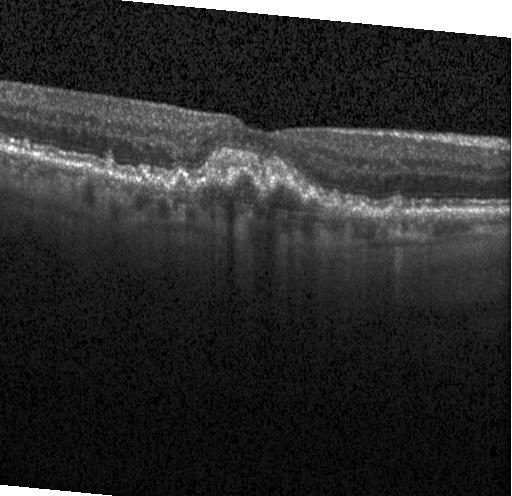
Retinal OCT cross-section showing choroidal neovascularization.